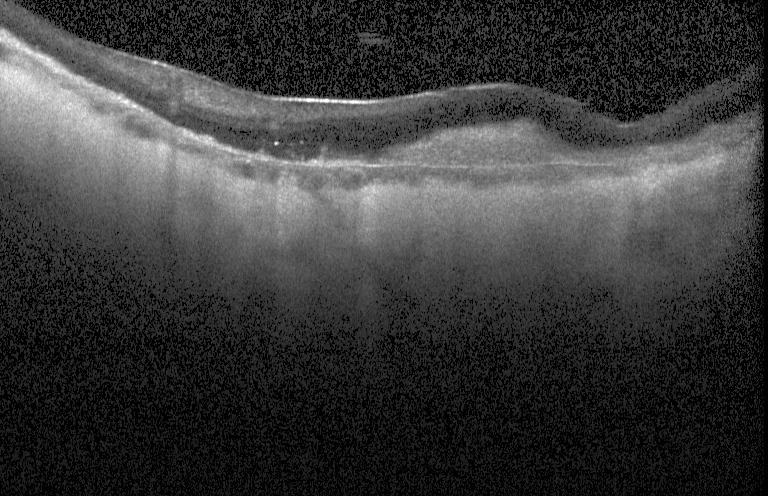

Through the macula; spectral-domain OCT; optical coherence tomography scan; Heidelberg Spectralis.
OCT finding: a choroidal neovascular membrane.